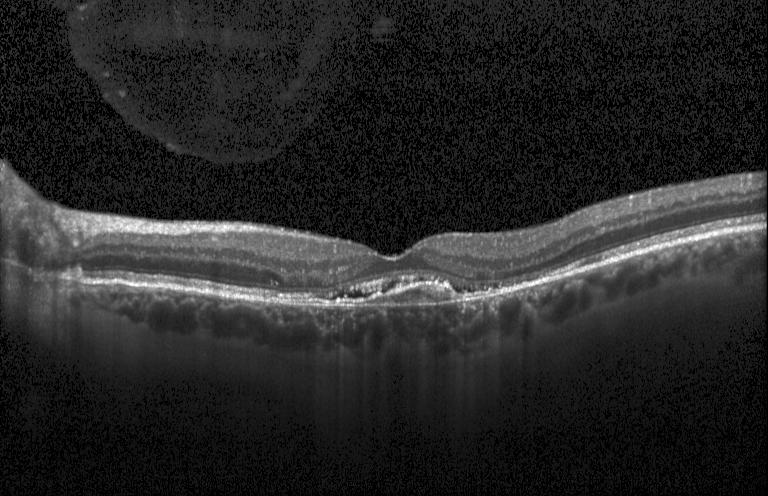

OCT B-scan showing a choroidal neovascular membrane.